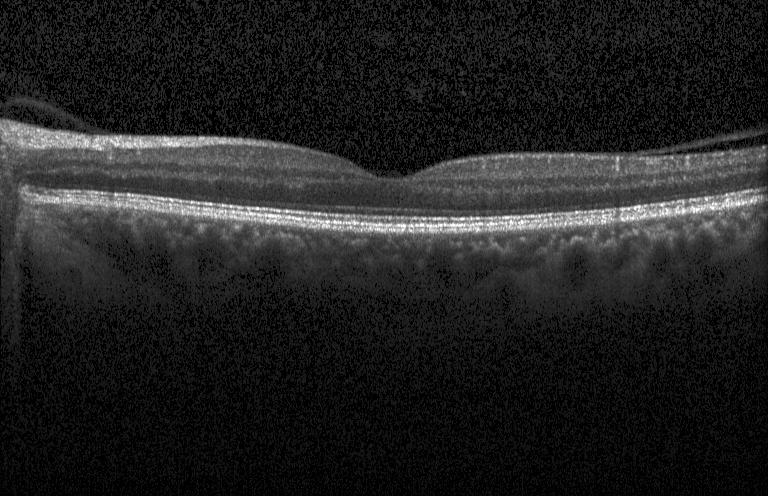
Spectral-domain optical coherence tomography; OCT B-scan — Impression: no evidence of choroidal neovascularization, diabetic macular edema, or drusen.